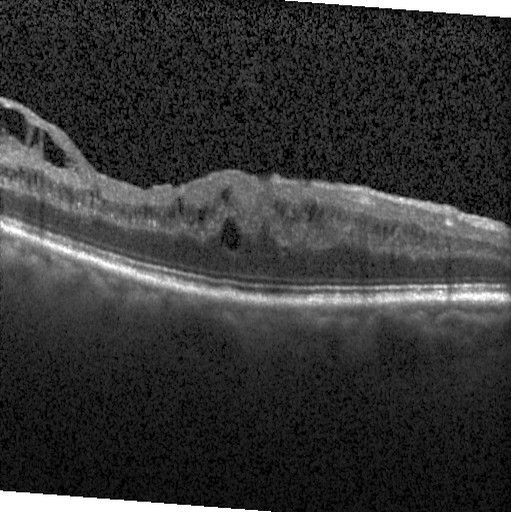
Optical coherence tomography scan — Finding: diabetic macular edema (DME).